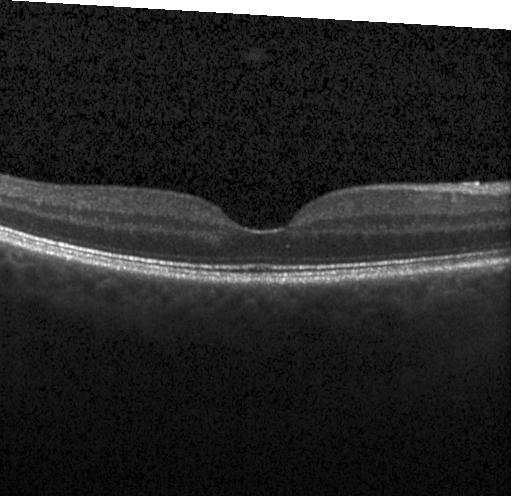 Spectral-domain OCT · instrument: Heidelberg Spectralis · optical coherence tomography B-scan · through the macula.
Neither CNV, DME, nor drusen.